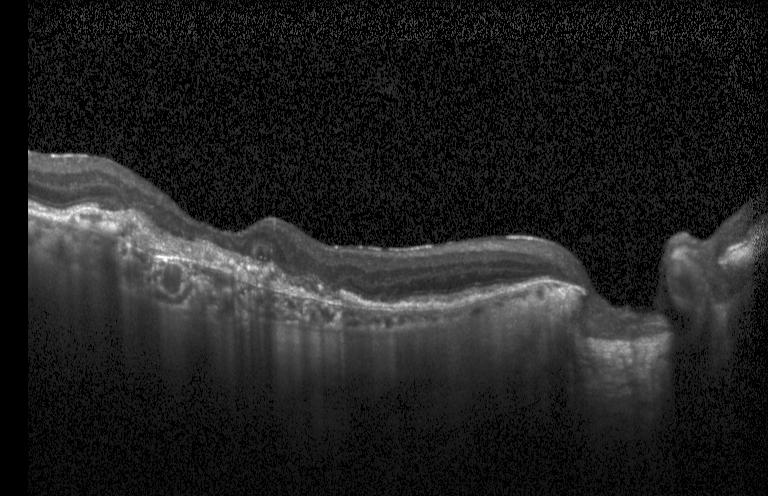

Impression: CNV.